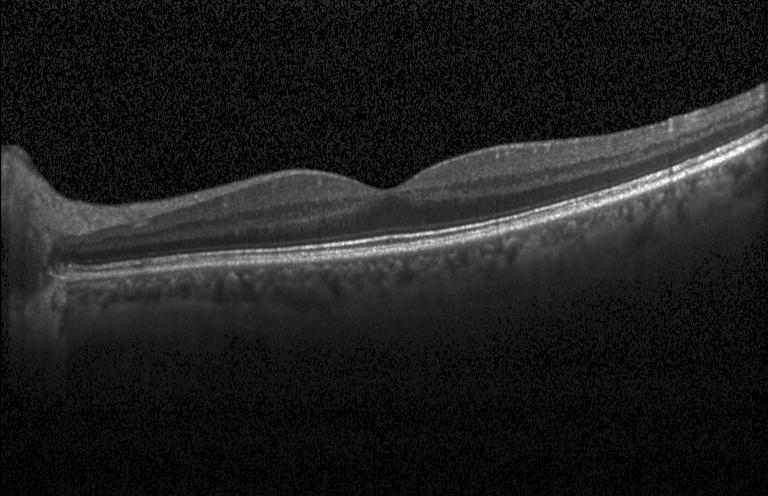

Finding: no choroidal neovascularization, no diabetic macular edema, and no drusen.